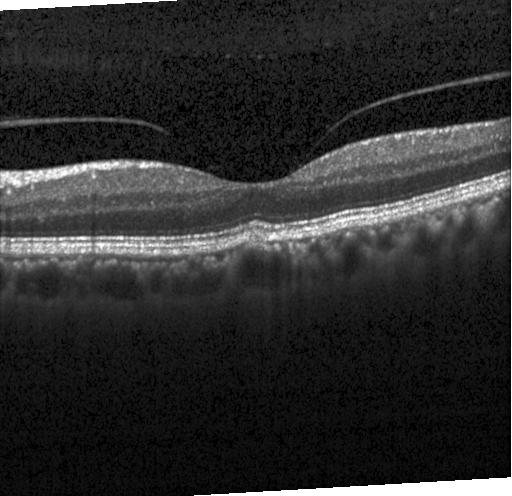
Instrument: Heidelberg Spectralis. SD-OCT. Optical coherence tomography B-scan. Macular scan — Finding: no choroidal neovascularization, no diabetic macular edema, and no drusen.